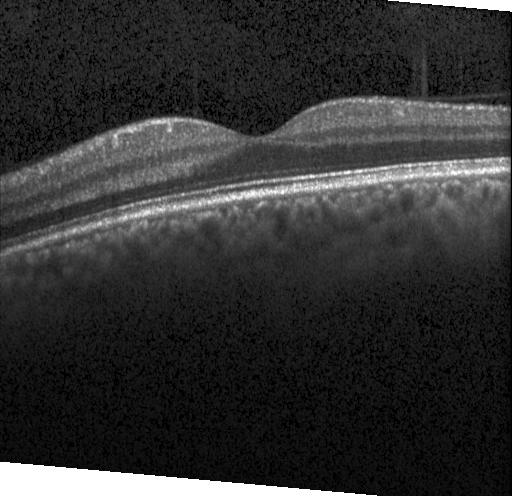
OCT scan showing no choroidal neovascularization, no diabetic macular edema, and no drusen.